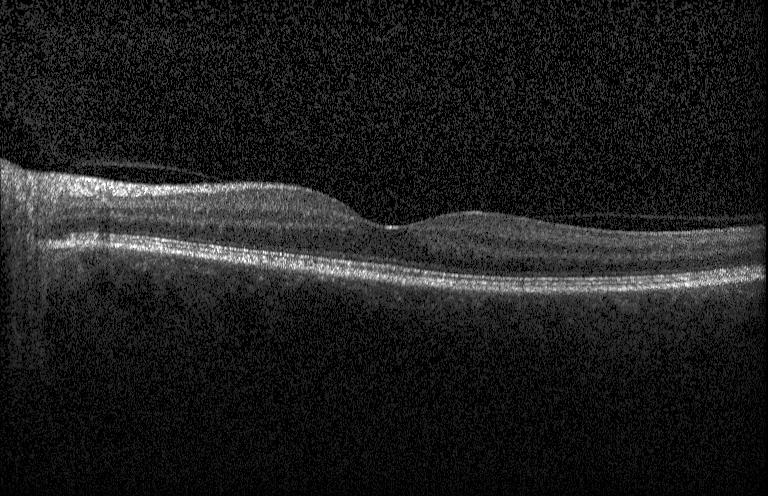

Heidelberg Spectralis OCT system · spectral-domain OCT · retinal OCT cross-section · horizontal scan through the fovea. This B-scan demonstrates neither choroidal neovascularization, diabetic macular edema, nor drusen.